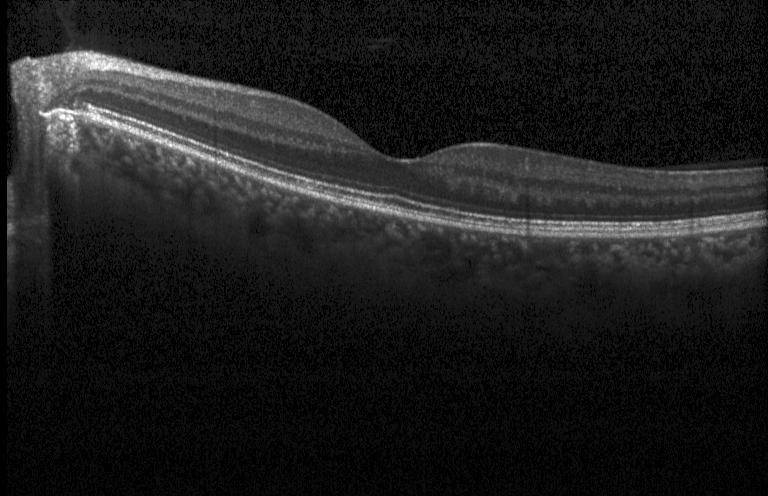 Optical coherence tomography scan
Impression: no choroidal neovascularization, diabetic macular edema, or drusen.